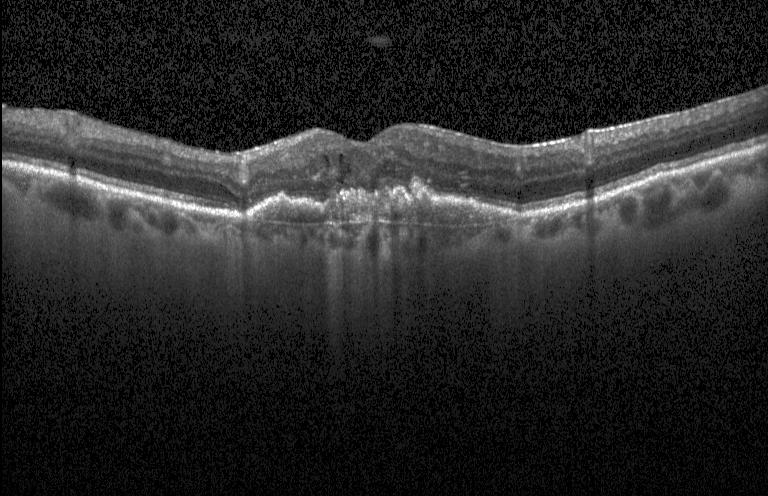
Spectral-domain OCT B-scan: a choroidal neovascular membrane.